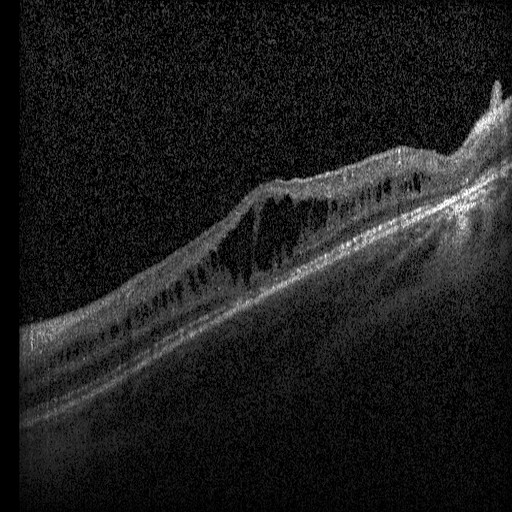

Spectral-domain OCT; Heidelberg Spectralis; optical coherence tomography scan. Dx: diabetic macular edema (DME).